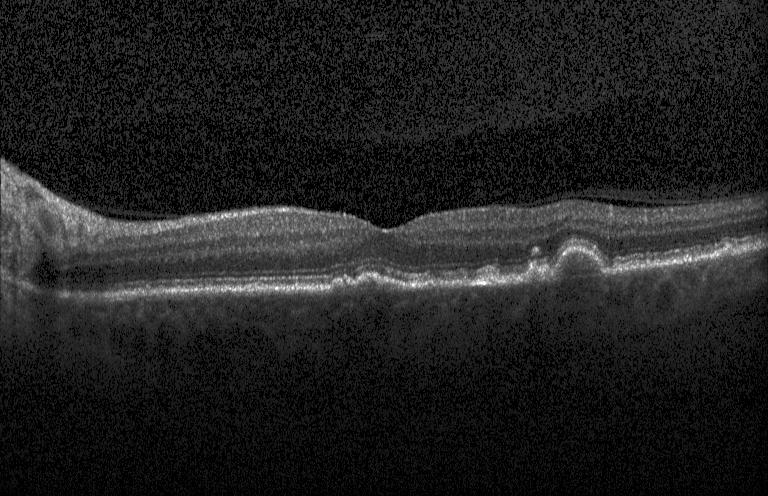
Diagnosis: sub-RPE drusenoid deposits.